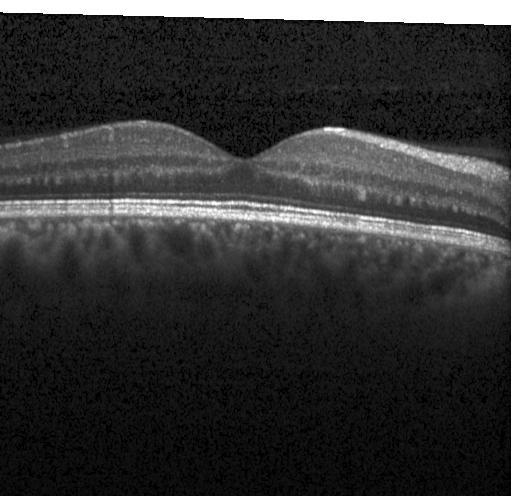

SD-OCT. Heidelberg Spectralis OCT system. Retinal OCT cross-section. Assessment: no choroidal neovascularization, diabetic macular edema, or drusen.